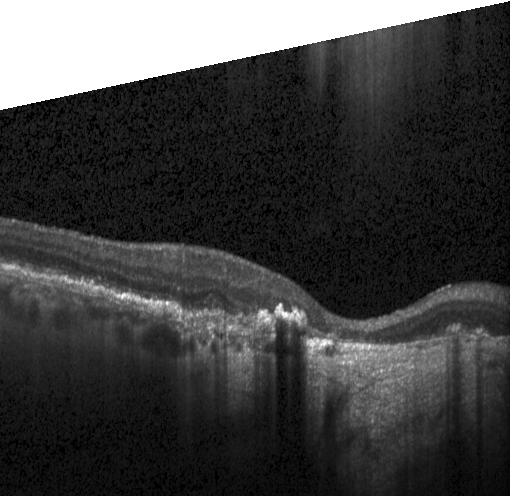
Optical coherence tomography scan · horizontal scan through the fovea · Heidelberg Spectralis OCT system · SD-OCT — Finding: choroidal neovascularization (CNV).